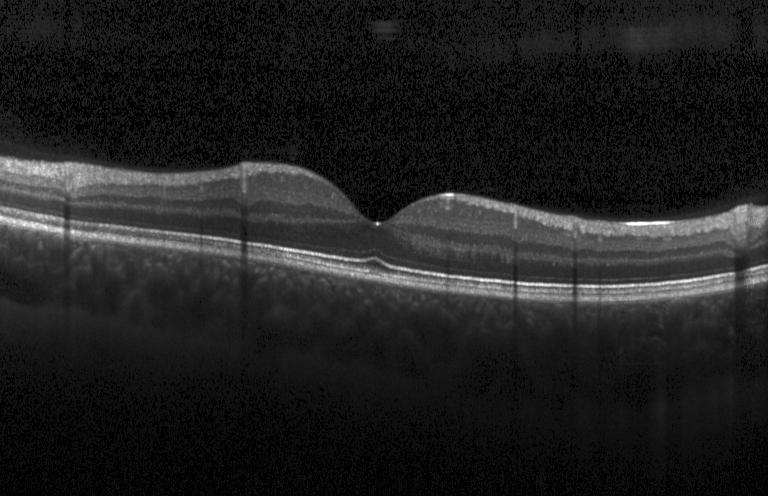
Heidelberg Spectralis; OCT line scan; SD-OCT
Neither CNV, DME, nor drusen.